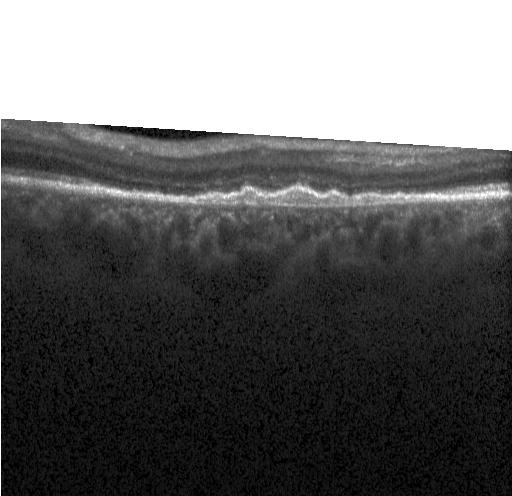

OCT B-scan; horizontal scan through the fovea; Heidelberg Spectralis; spectral-domain optical coherence tomography
Impression: choroidal neovascularization (CNV).